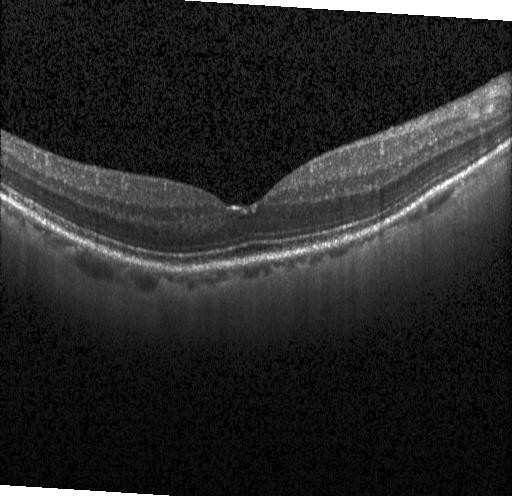

Acquired on a Heidelberg Spectralis; spectral-domain OCT; fovea-centered; OCT B-scan
Impression: neither choroidal neovascularization, diabetic macular edema, nor drusen.